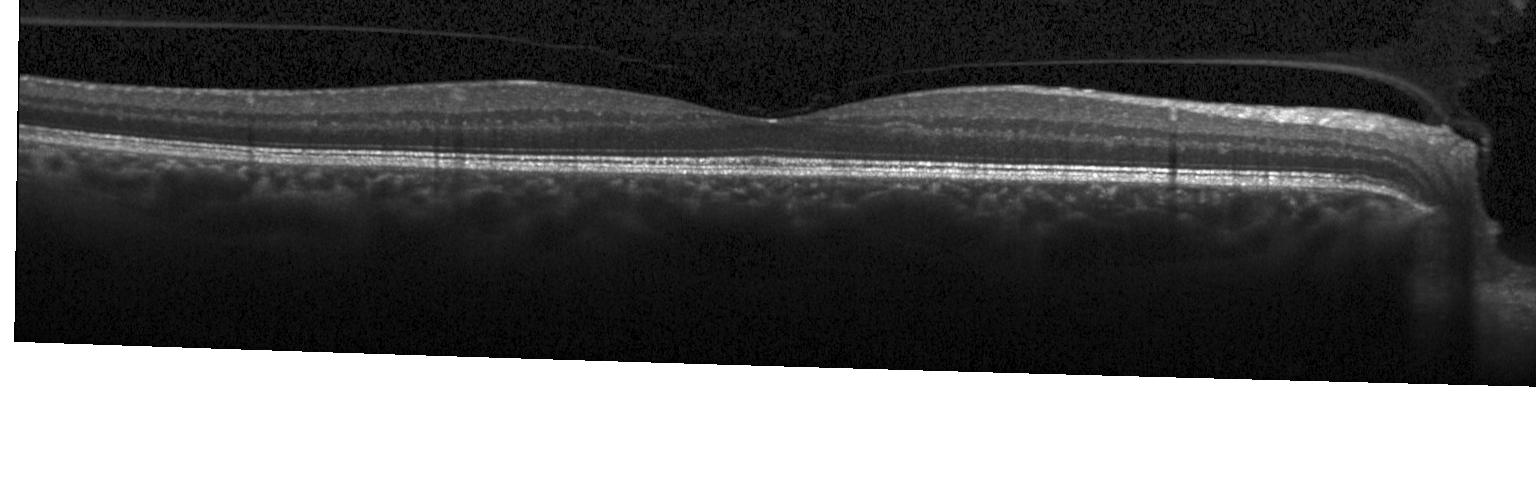
SD-OCT · optical coherence tomography scan · Heidelberg Spectralis
Assessment: neither CNV, DME, nor drusen.